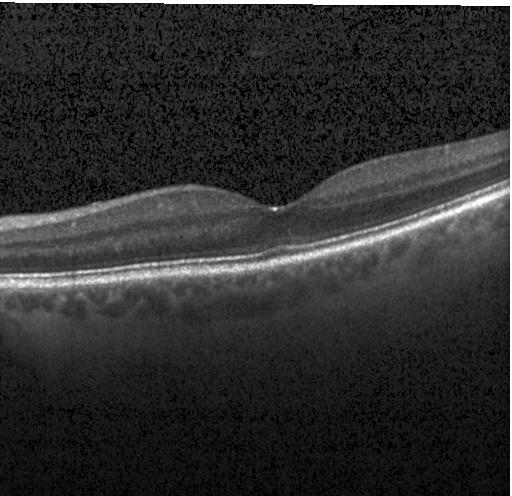 Finding: no choroidal neovascularization, no diabetic macular edema, and no drusen.